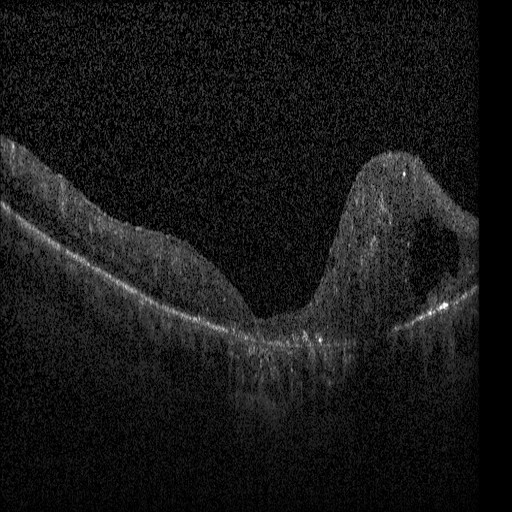

Diagnosis: diabetic macular edema.